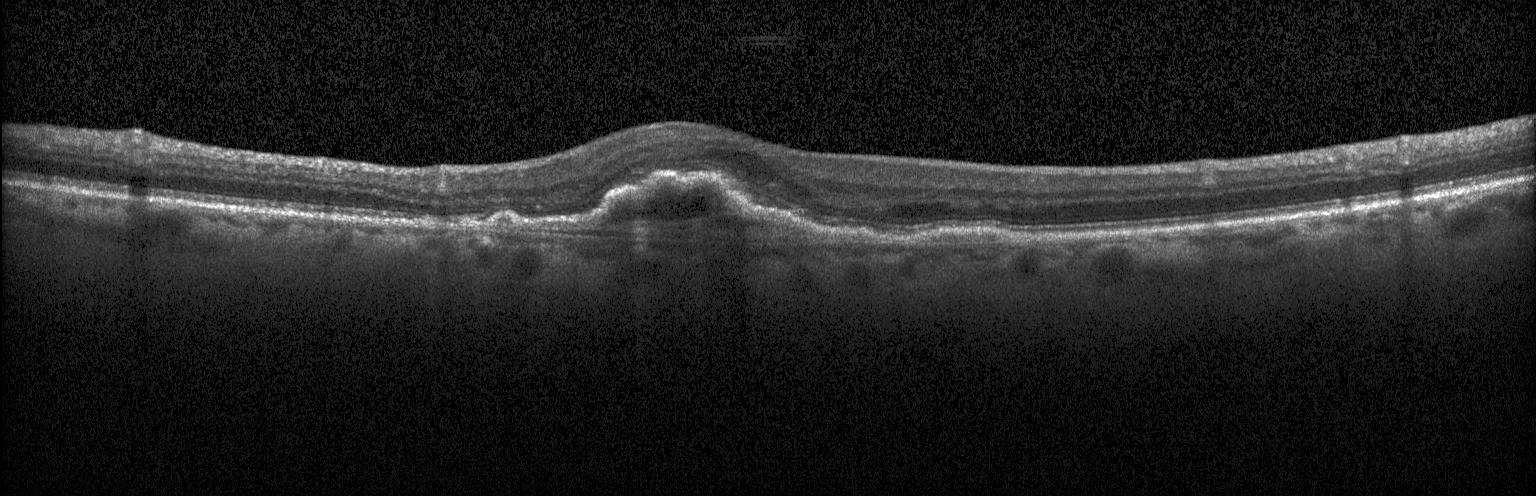

OCT B-scan; Heidelberg Spectralis OCT system; spectral-domain OCT — Impression: a choroidal neovascular membrane.